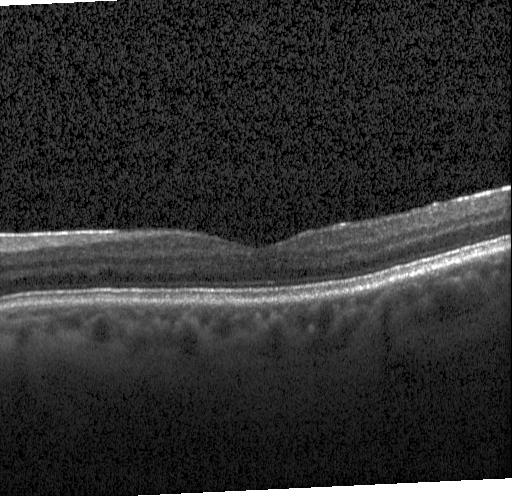

Diagnosis: no evidence of choroidal neovascularization, diabetic macular edema, or drusen.